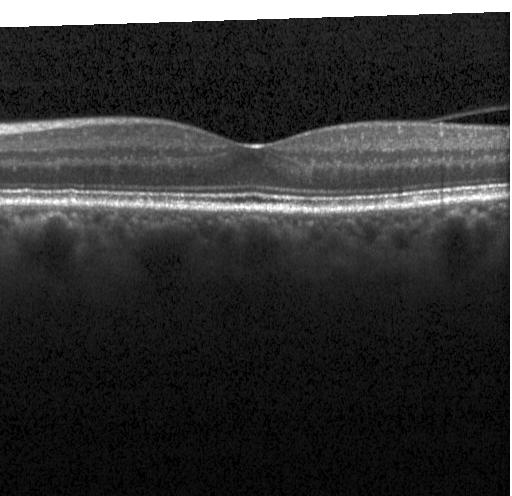 Finding: no CNV, no DME, and no drusen.